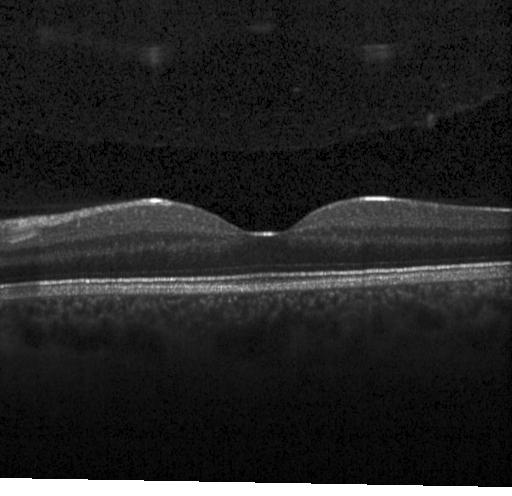 Neither choroidal neovascularization, diabetic macular edema, nor drusen.